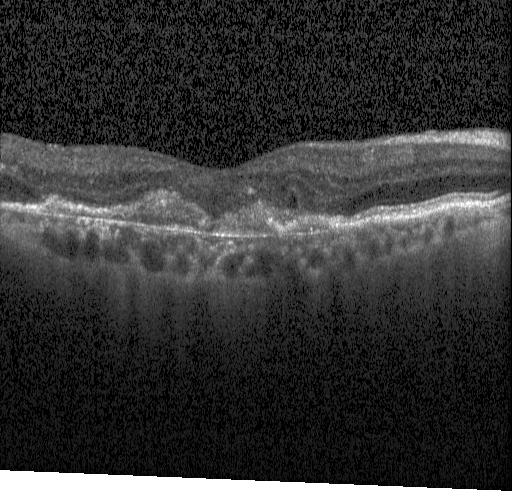

Horizontal scan through the fovea, OCT line scan, spectral-domain OCT
This B-scan demonstrates a choroidal neovascular membrane.